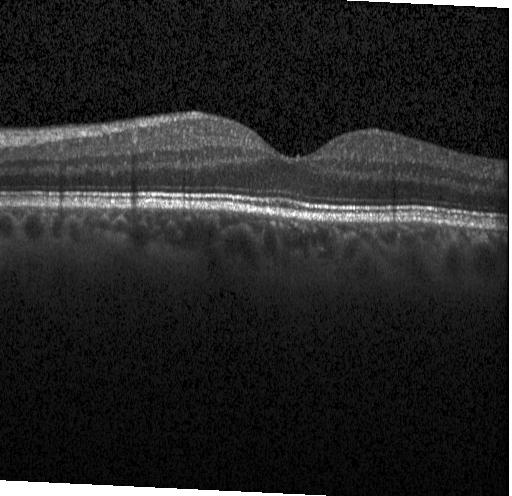
Spectral-domain OCT. Instrument: Heidelberg Spectralis. Fovea-centered. Retinal OCT B-scan
Impression: no choroidal neovascularization, diabetic macular edema, or drusen.